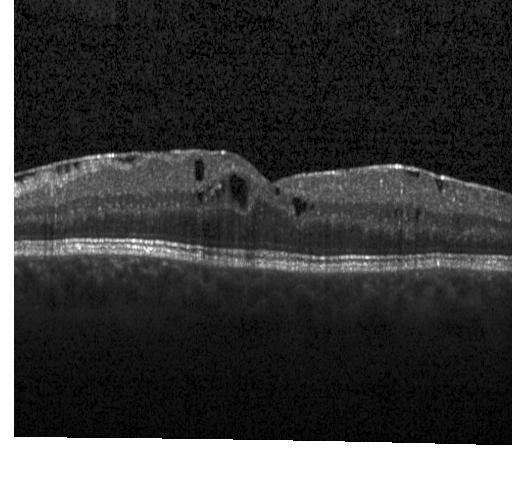 Optical coherence tomography B-scan. Spectral-domain OCT. Impression: diabetic macular edema (DME).